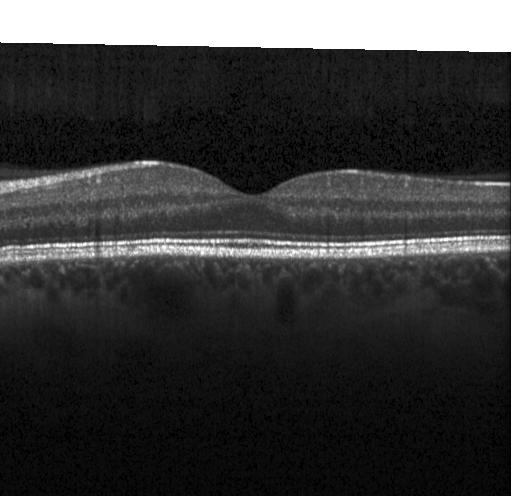

Dx: no choroidal neovascularization, diabetic macular edema, or drusen.